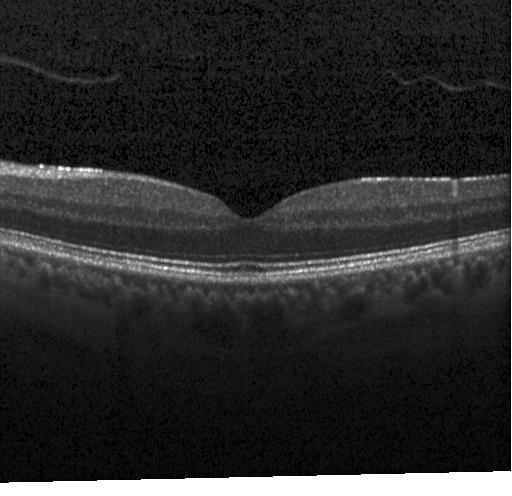

Macular OCT: neither choroidal neovascularization, diabetic macular edema, nor drusen.